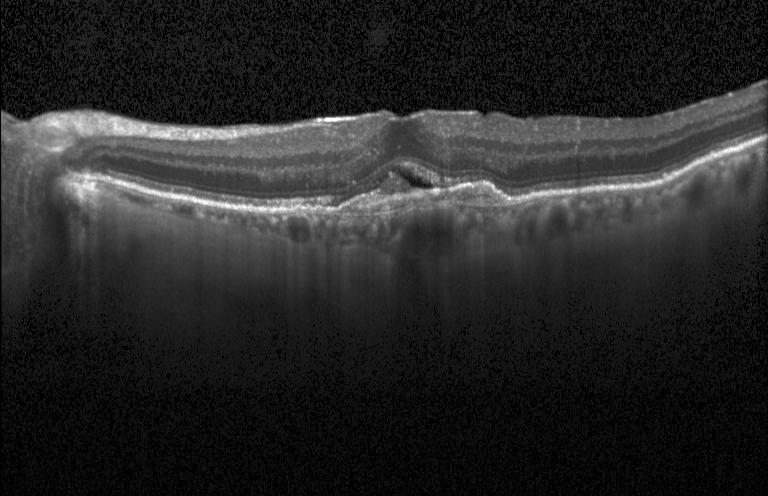 Macular OCT demonstrating a choroidal neovascular membrane.